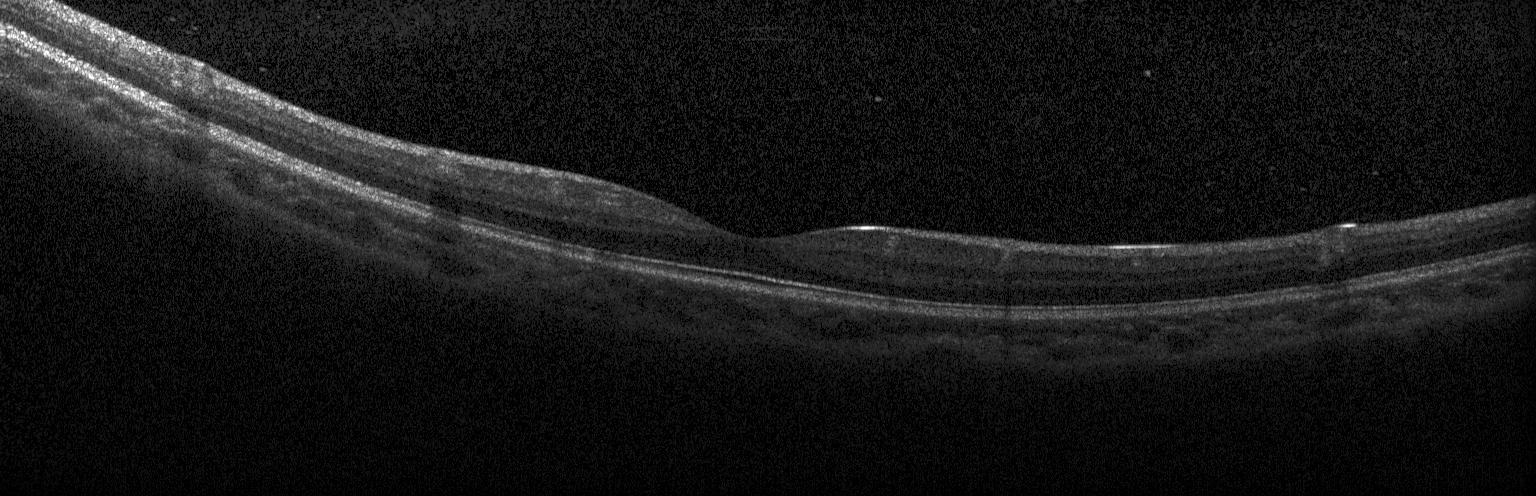

The scan shows neither choroidal neovascularization, diabetic macular edema, nor drusen.